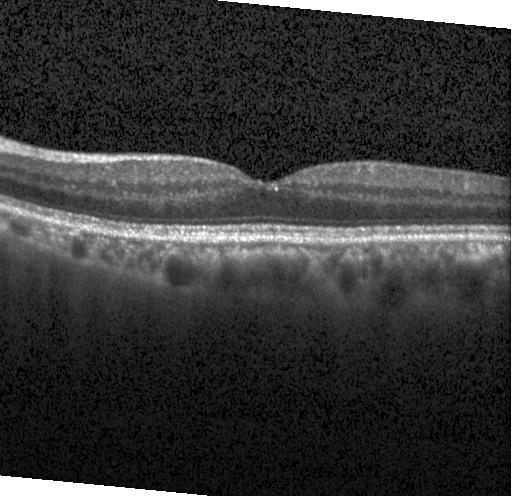 The scan shows neither choroidal neovascularization, diabetic macular edema, nor drusen.